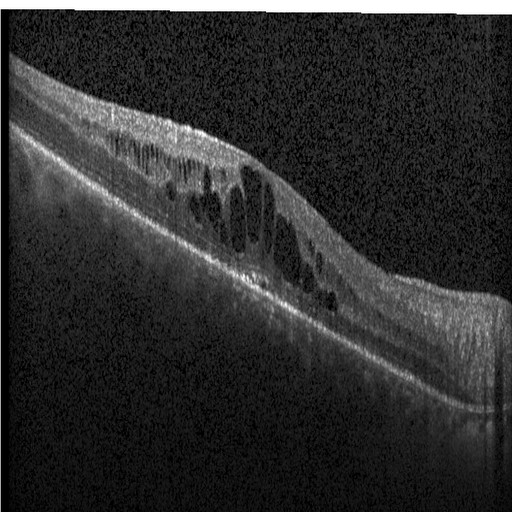 Optical coherence tomography B-scan
Impression: diabetic macular edema (DME).